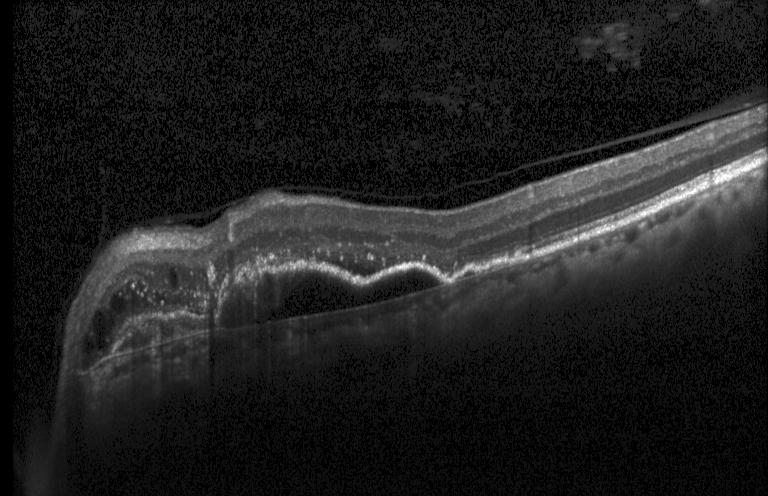
Finding: a choroidal neovascular membrane.